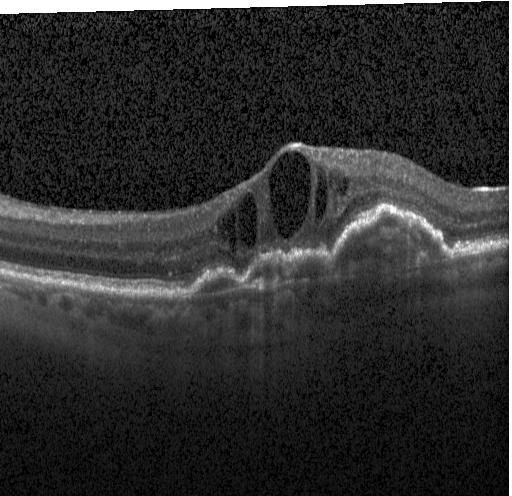 Centered on the fovea, retinal OCT cross-section — Assessment: choroidal neovascularization.